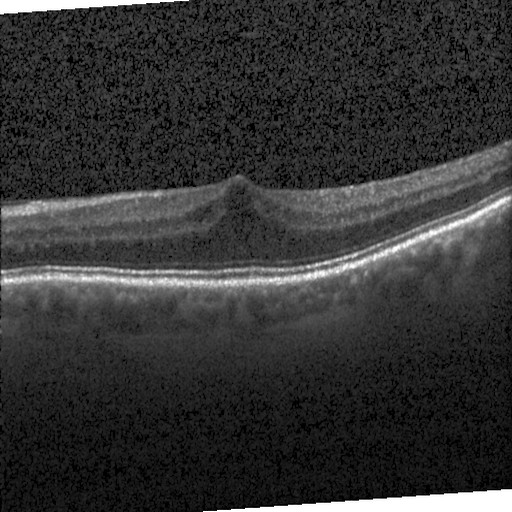
Spectral-domain OCT. Acquired on a Heidelberg Spectralis. Retinal OCT B-scan. Through the macula.
Impression: diabetic macular edema (DME).